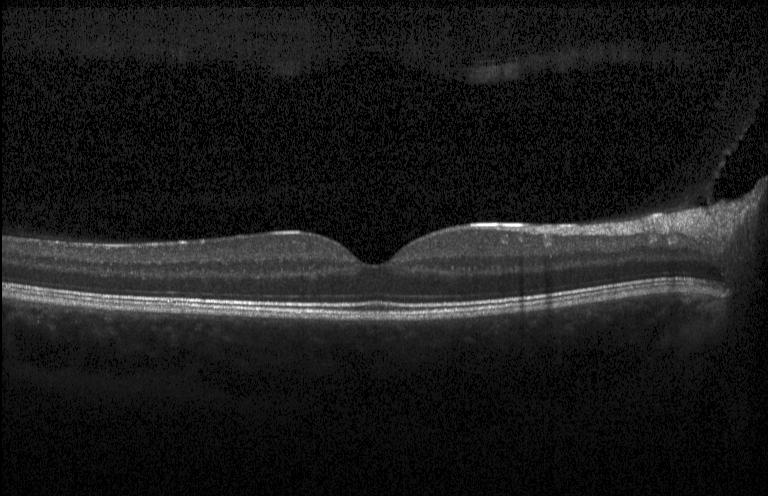

Optical coherence tomography B-scan
Finding: no evidence of CNV, DME, or drusen.